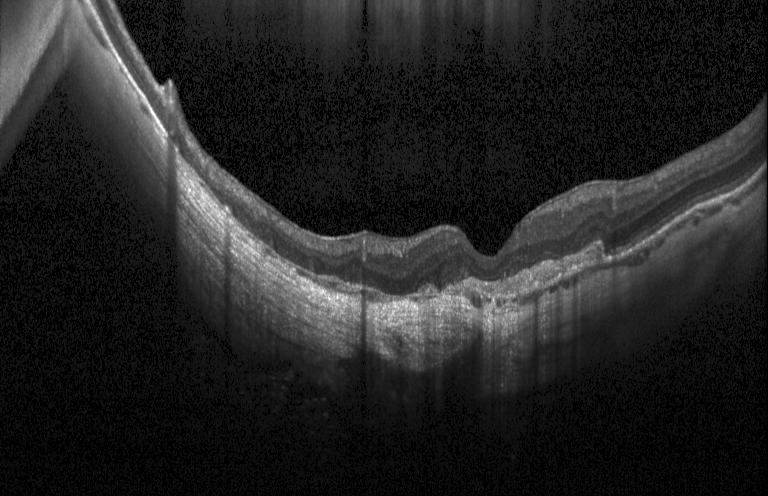
Optical coherence tomography scan, spectral-domain optical coherence tomography — Diagnosis: choroidal neovascularization.